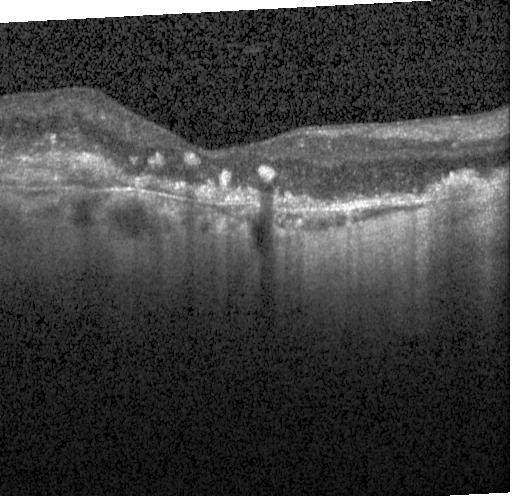
This B-scan demonstrates a choroidal neovascular membrane.